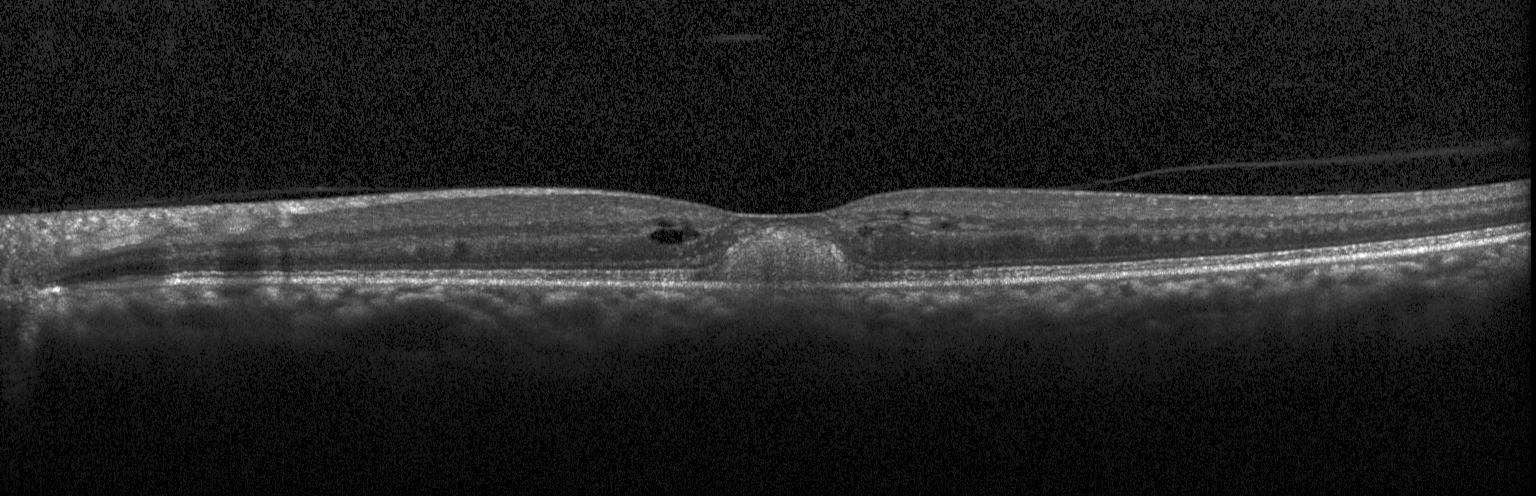 OCT line scan — The scan shows choroidal neovascularization.